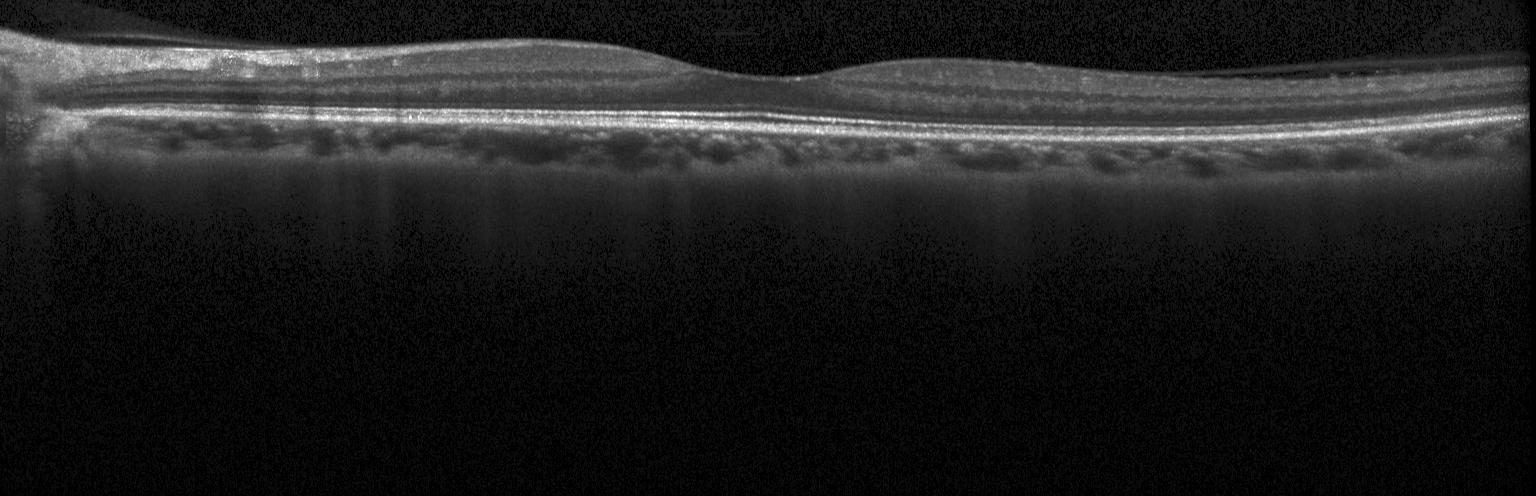
Impression: no evidence of CNV, DME, or drusen.